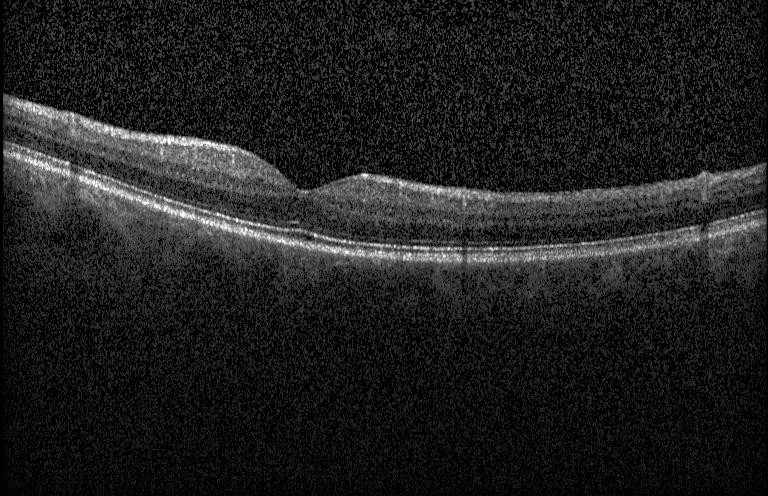 OCT line scan.
Impression: no evidence of CNV, DME, or drusen.